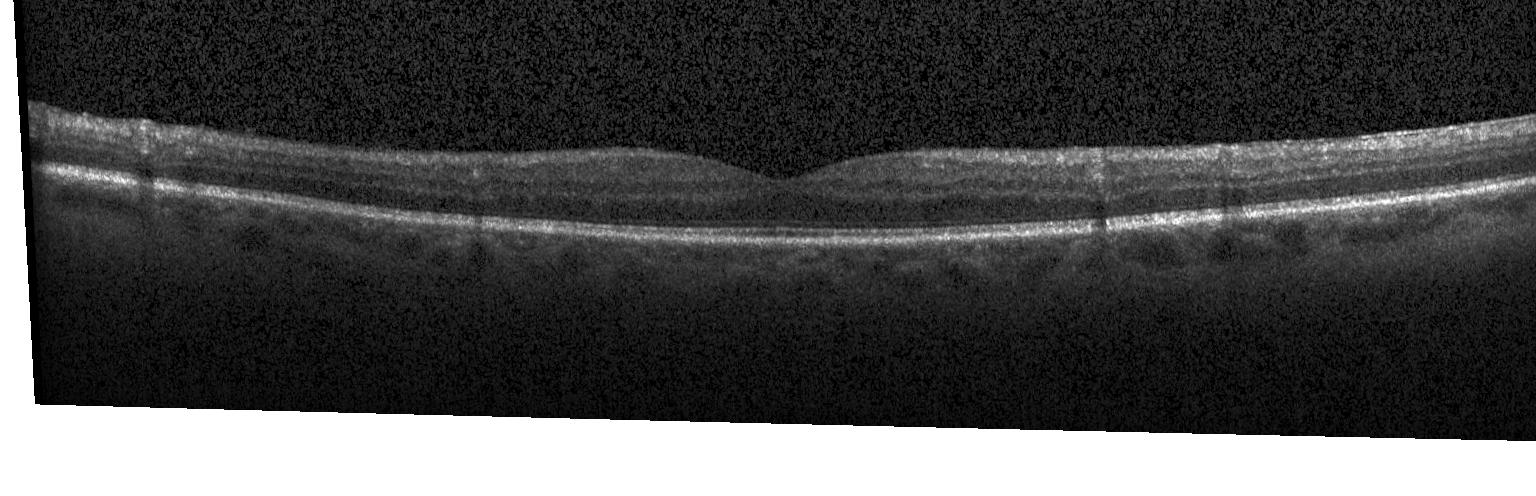 OCT finding: no choroidal neovascularization, no diabetic macular edema, and no drusen.